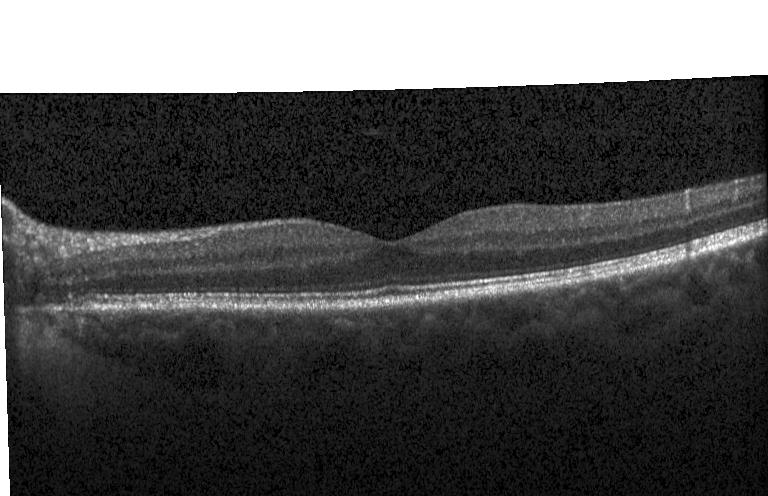

Finding: neither choroidal neovascularization, diabetic macular edema, nor drusen.